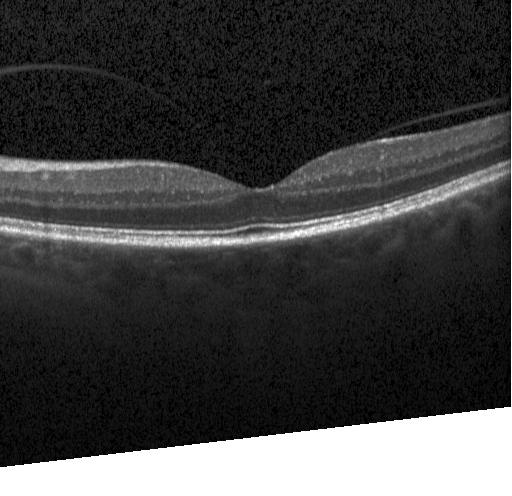
Dx: neither CNV, DME, nor drusen.